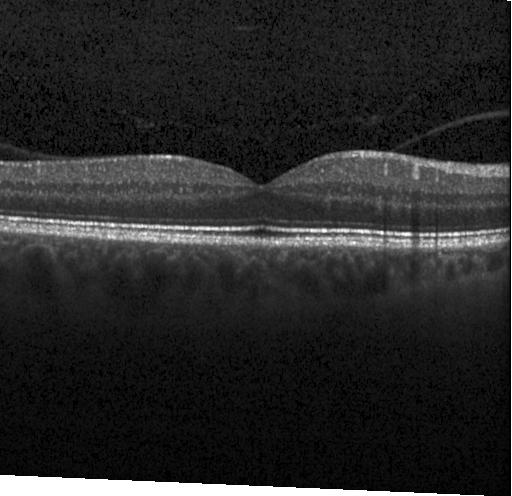 Retinal OCT cross-section; Heidelberg Spectralis — Finding: no choroidal neovascularization, diabetic macular edema, or drusen.